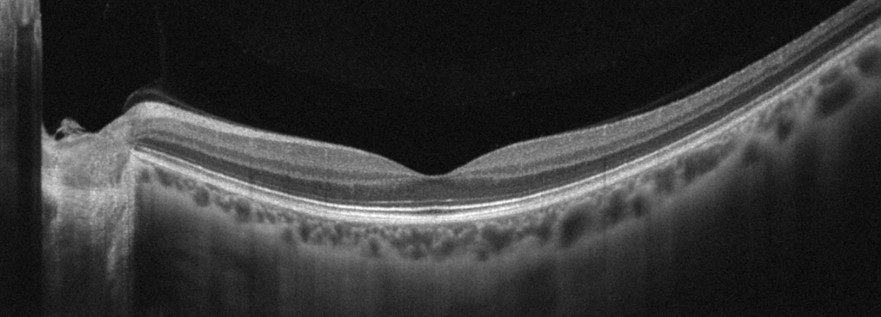

Impression: absence of AMD, DME, ERM, RAO, RVO, and vitreomacular interface disease.